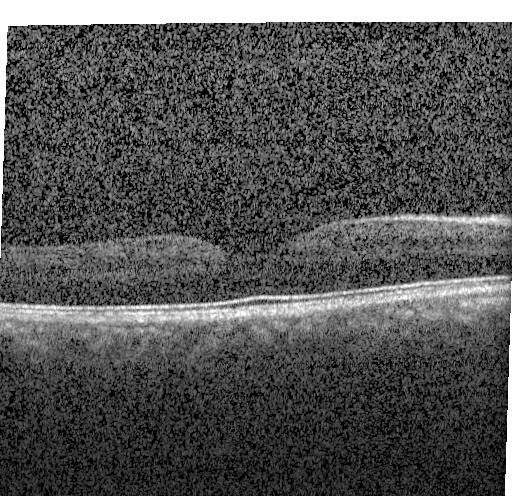
Through the macula, retinal OCT B-scan, SD-OCT, acquired on a Heidelberg Spectralis
The scan shows no choroidal neovascularization, diabetic macular edema, or drusen.